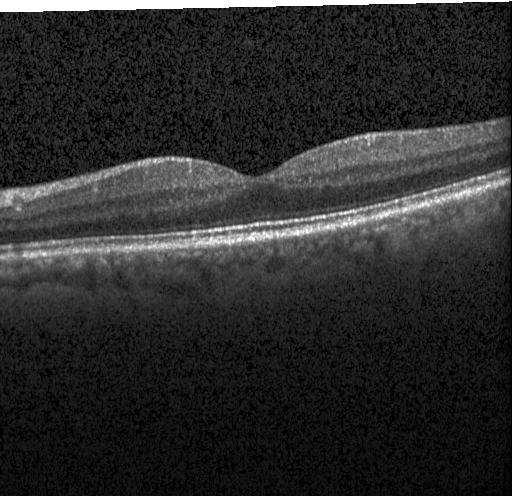
SD-OCT · retinal OCT cross-section — The scan shows no evidence of choroidal neovascularization, diabetic macular edema, or drusen.